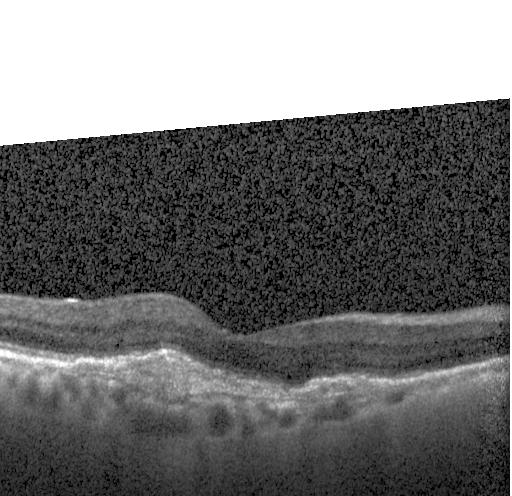 Instrument: Heidelberg Spectralis · retinal OCT cross-section · horizontal scan through the fovea · spectral-domain OCT — The scan shows a choroidal neovascular membrane.